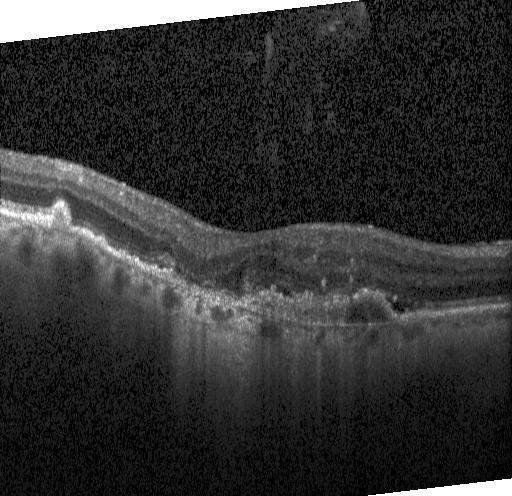

CNV.